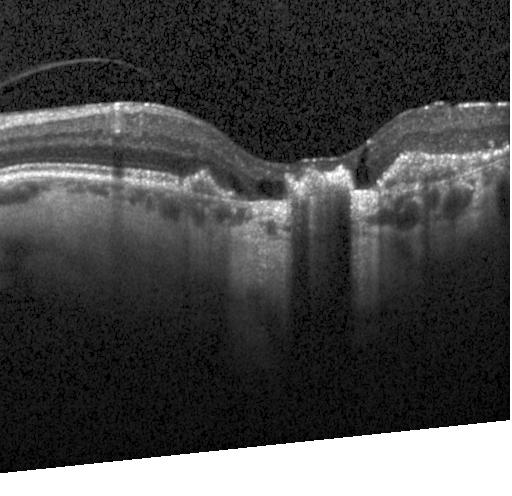

OCT line scan
This B-scan demonstrates CNV.